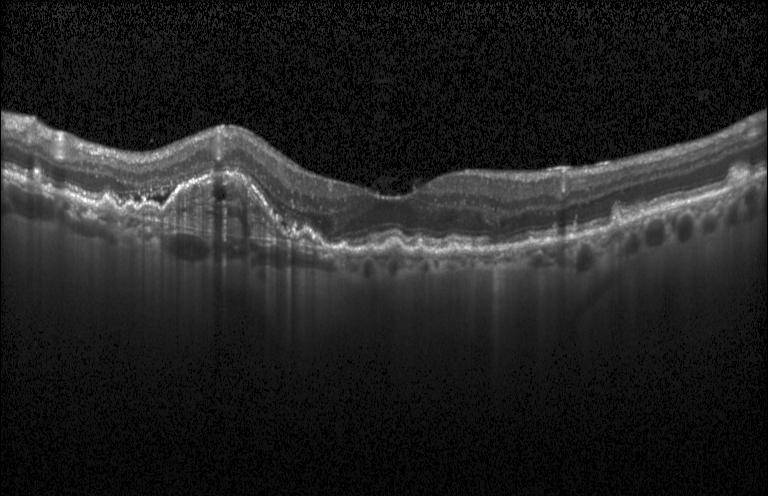 Optical coherence tomography B-scan; instrument: Heidelberg Spectralis; fovea-centered.
Diagnosis: choroidal neovascularization (CNV).